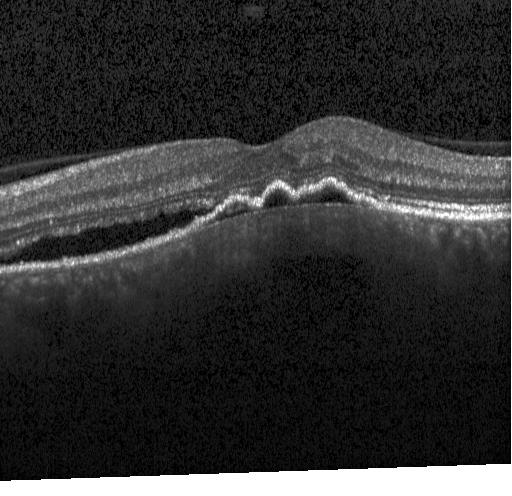
Centered on the fovea. OCT line scan. Heidelberg Spectralis — A choroidal neovascular membrane.